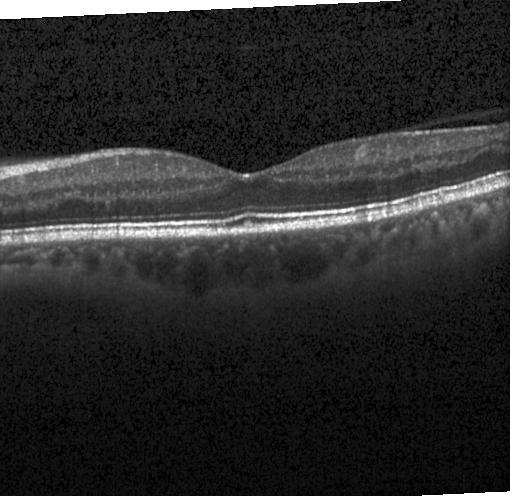

Diagnosis: no evidence of choroidal neovascularization, diabetic macular edema, or drusen.